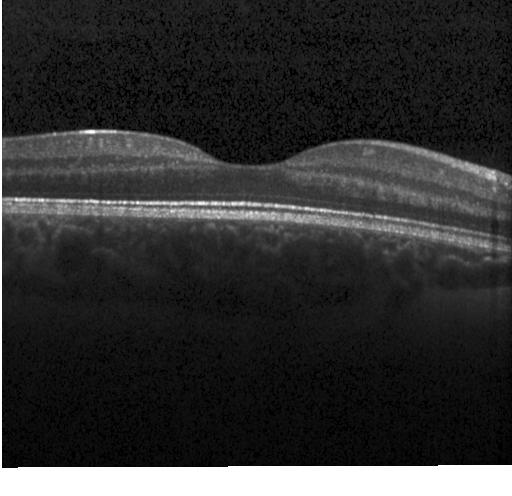 Assessment: no choroidal neovascularization, diabetic macular edema, or drusen.